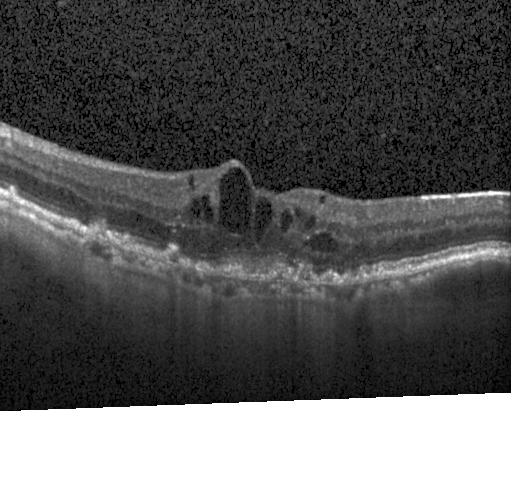

Retinal OCT B-scan. Acquired on a Heidelberg Spectralis. Assessment: a choroidal neovascular membrane.